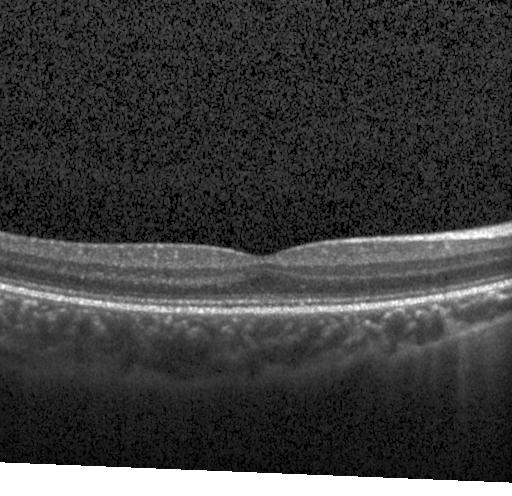

Centered on the fovea; retinal OCT B-scan
The scan shows no evidence of CNV, DME, or drusen.